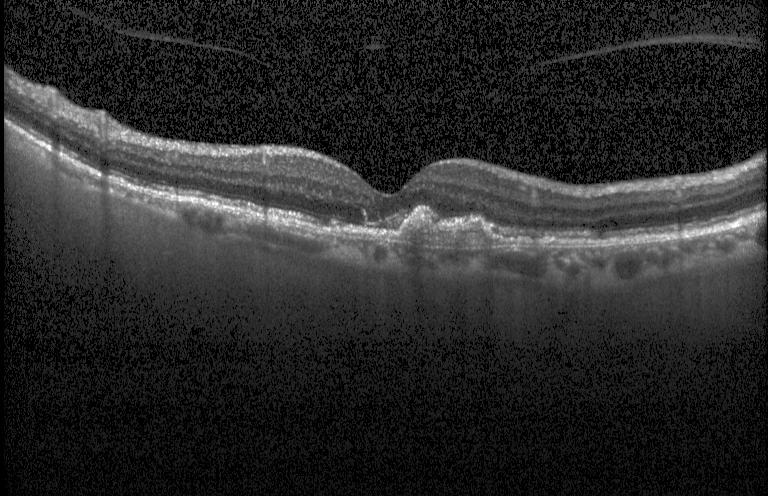

Spectral-domain OCT; retinal OCT cross-section; centered on the fovea — Dx: a choroidal neovascular membrane.